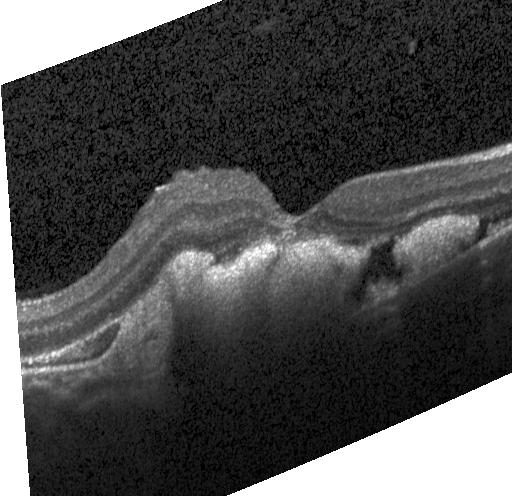 The scan shows a choroidal neovascular membrane.